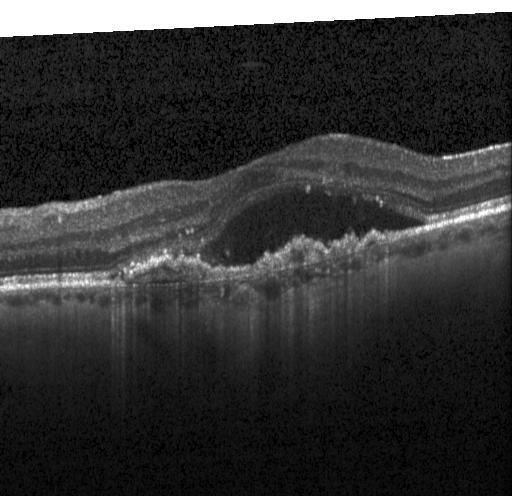

Optical coherence tomography scan, instrument: Heidelberg Spectralis, fovea-centered
Impression: CNV.